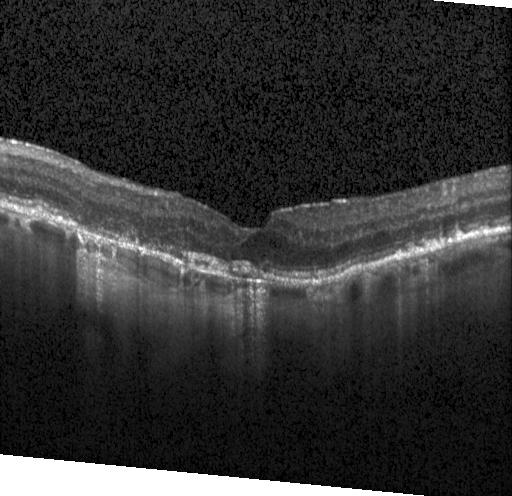

Spectral-domain optical coherence tomography · OCT B-scan · centered on the fovea · instrument: Heidelberg Spectralis. Diagnosis: neither CNV, DME, nor drusen.